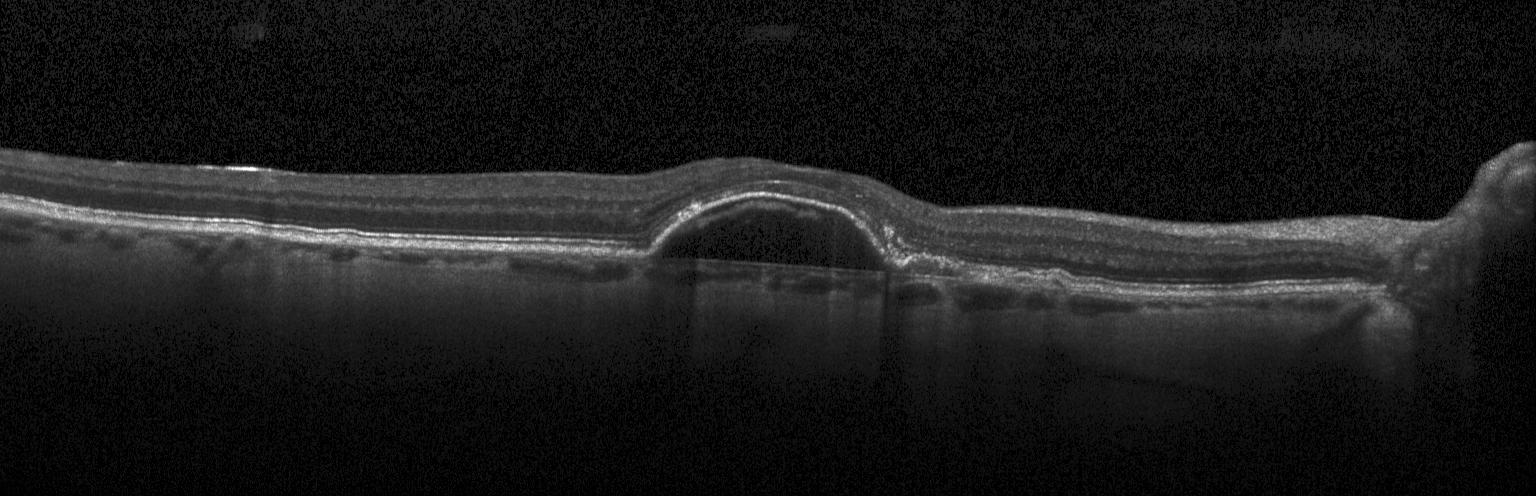 Spectral-domain OCT · horizontal scan through the fovea · Heidelberg Spectralis OCT system · OCT line scan. Choroidal neovascularization (CNV).